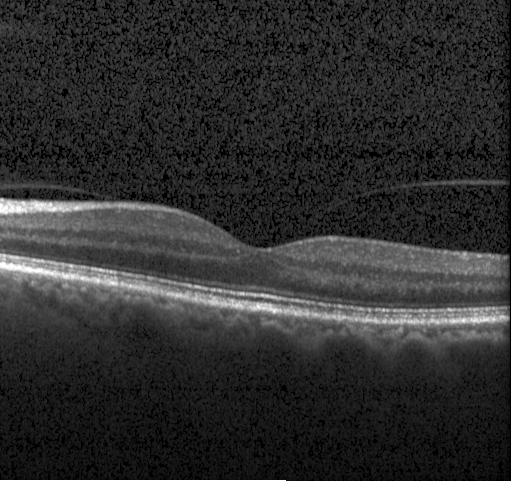

Macular scan · optical coherence tomography B-scan
Dx: neither CNV, DME, nor drusen.